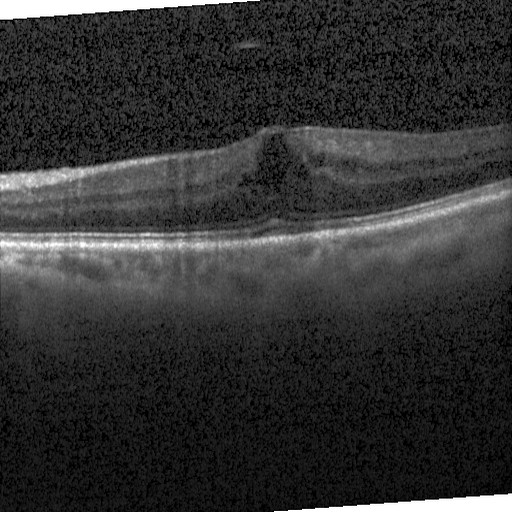

OCT B-scan — Impression: diabetic macular edema (DME).